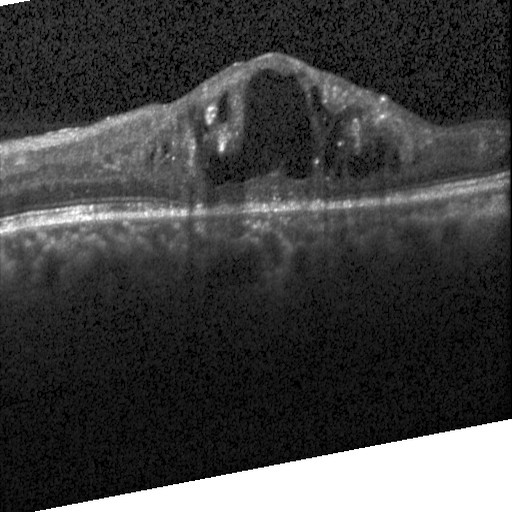

Optical coherence tomography scan; spectral-domain OCT; instrument: Heidelberg Spectralis
Diagnosis: diabetic macular edema.